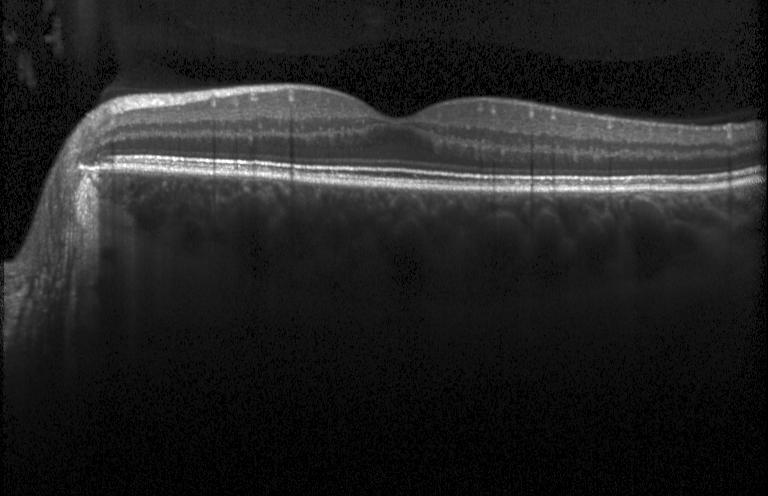 Optical coherence tomography scan. Heidelberg Spectralis. Macular OCT: no CNV, DME, or drusen.